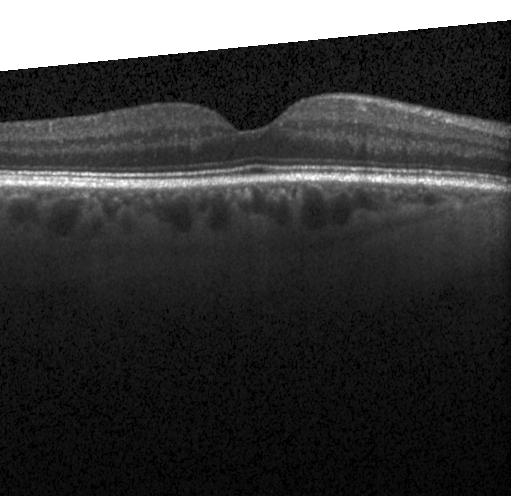 Assessment: no evidence of choroidal neovascularization, diabetic macular edema, or drusen.